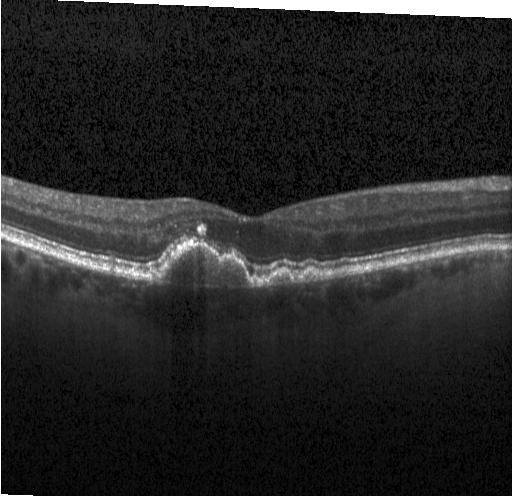 Retinal OCT B-scan
This B-scan demonstrates CNV.